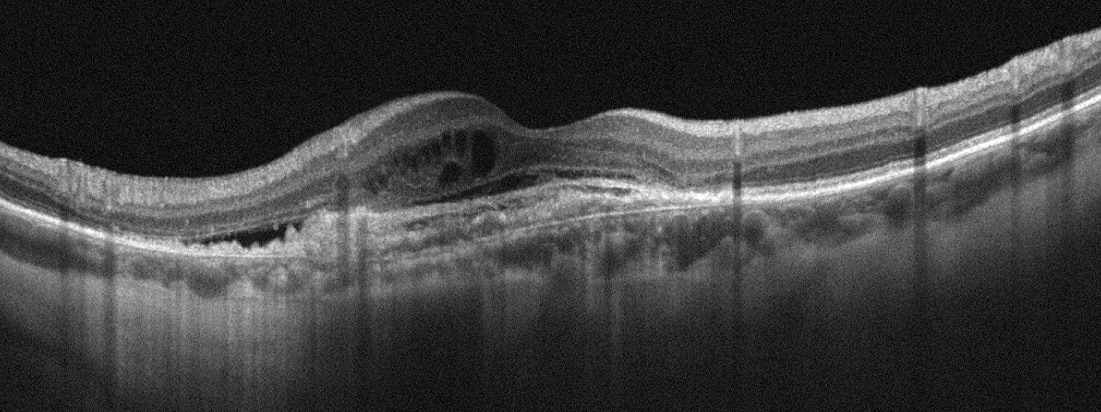
Dx: age-related macular degeneration.